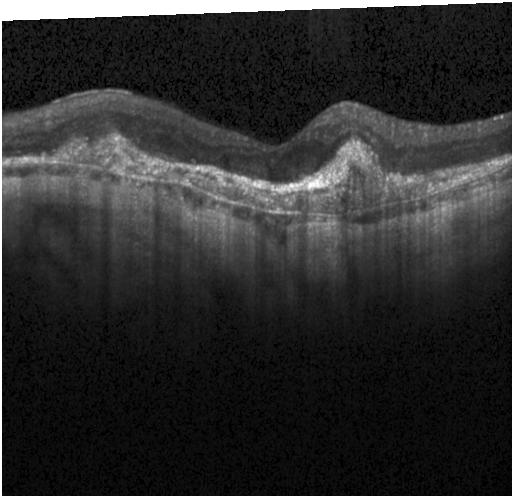 Through the macula, retinal OCT B-scan, instrument: Heidelberg Spectralis — Finding: a choroidal neovascular membrane.